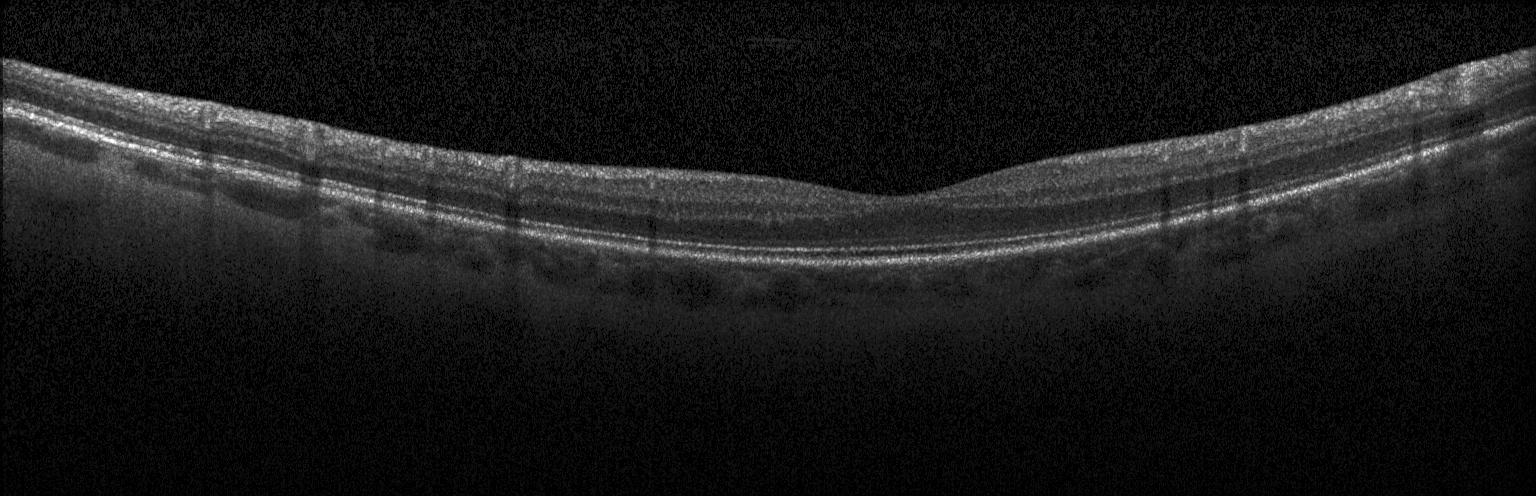 OCT scan showing no choroidal neovascularization, no diabetic macular edema, and no drusen.